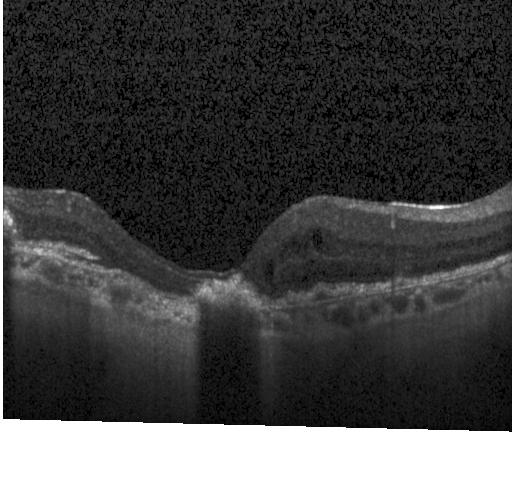 OCT B-scan; through the macula.
This B-scan demonstrates a choroidal neovascular membrane.